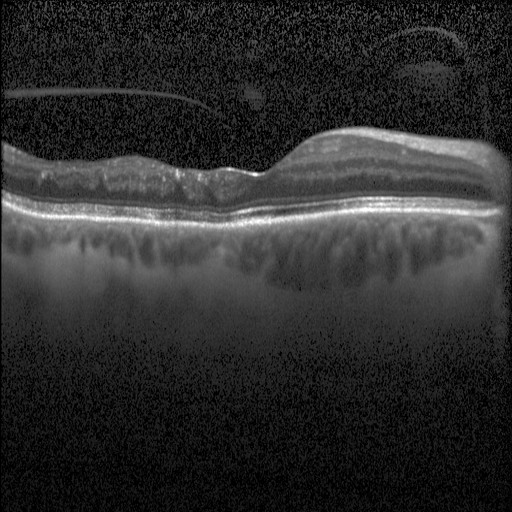 Through the macula, spectral-domain OCT, retinal OCT B-scan, acquired on a Heidelberg Spectralis.
Assessment: diabetic macular edema.